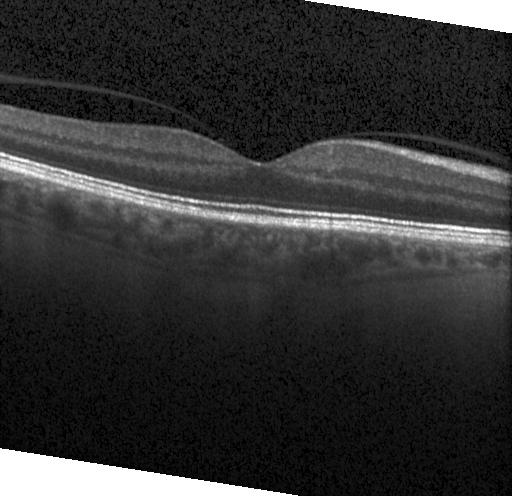

Acquired on a Heidelberg Spectralis, OCT line scan. This B-scan demonstrates no choroidal neovascularization, no diabetic macular edema, and no drusen.